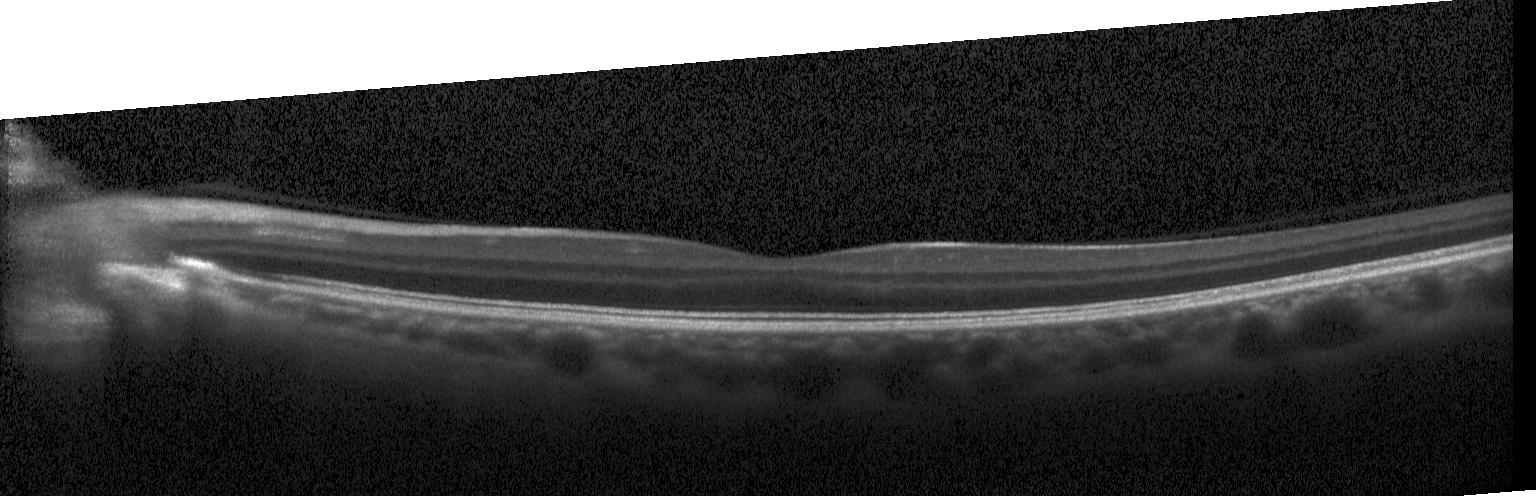 Macular OCT: no evidence of choroidal neovascularization, diabetic macular edema, or drusen.